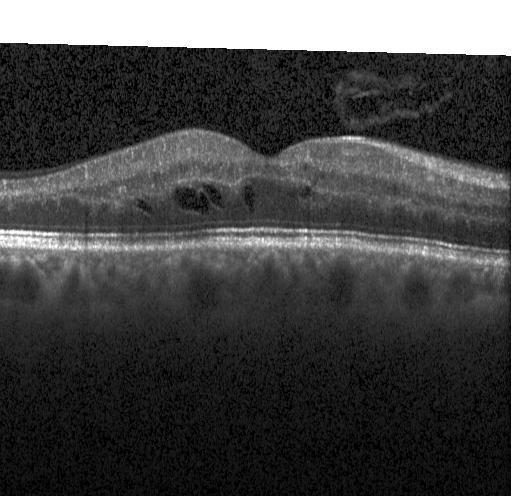
OCT B-scan showing diabetic macular edema.